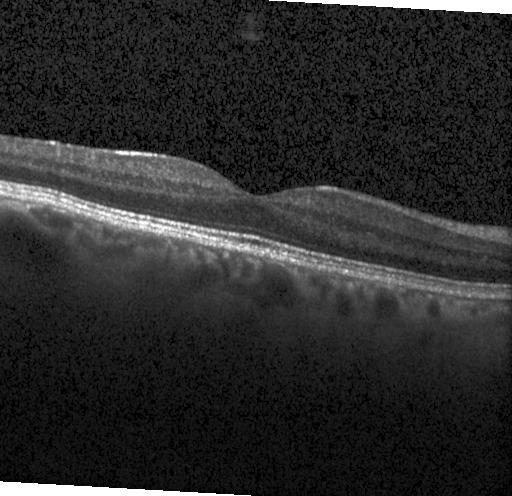 Optical coherence tomography scan
Diagnosis: no evidence of choroidal neovascularization, diabetic macular edema, or drusen.